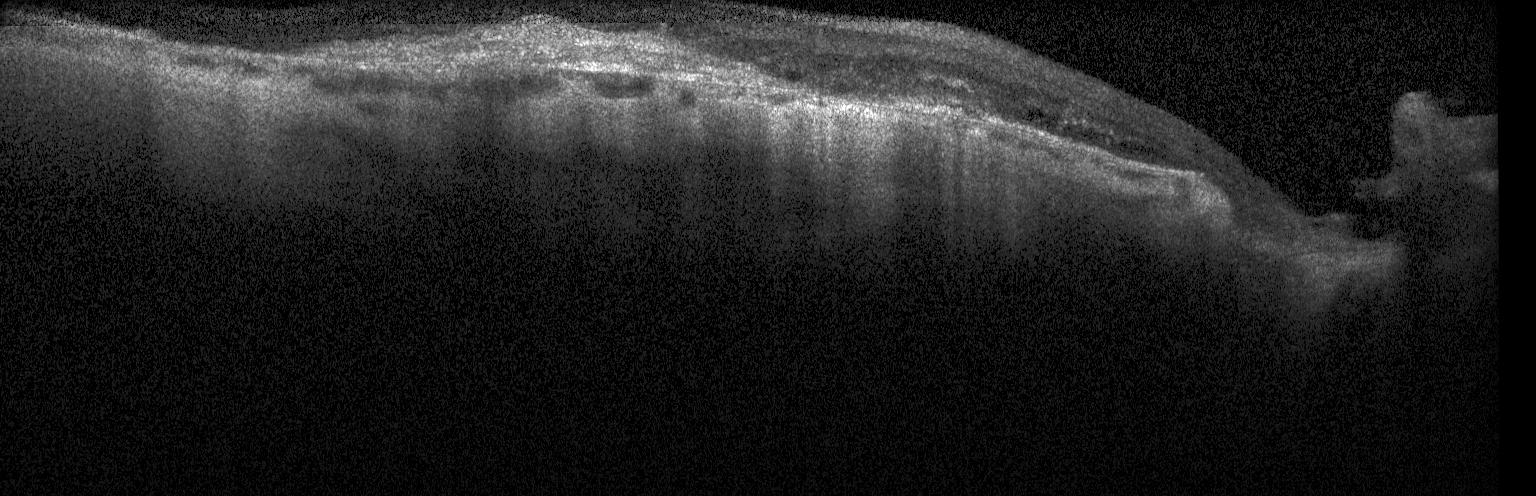
Optical coherence tomography B-scan; instrument: Heidelberg Spectralis. Diagnosis: a choroidal neovascular membrane.